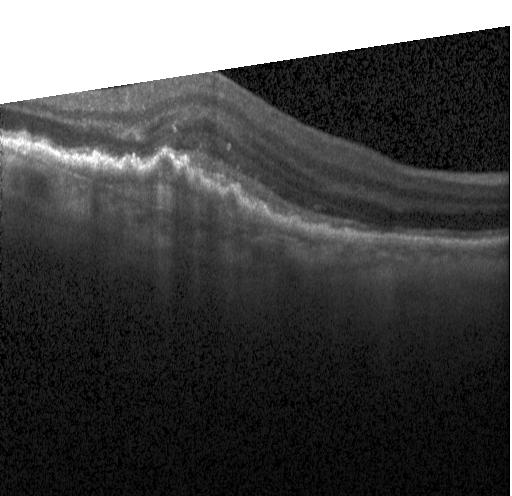 Retinal OCT cross-section, spectral-domain OCT, macular scan — Macular OCT: a choroidal neovascular membrane.